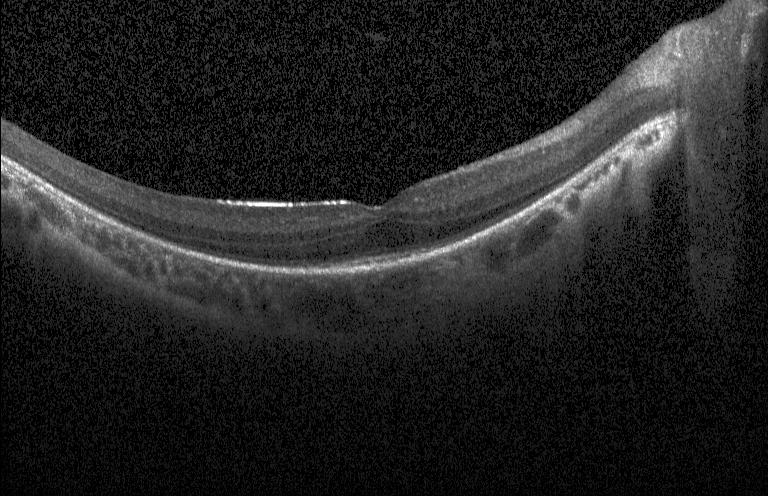 Spectral-domain OCT; OCT line scan; instrument: Heidelberg Spectralis — No choroidal neovascularization, diabetic macular edema, or drusen.